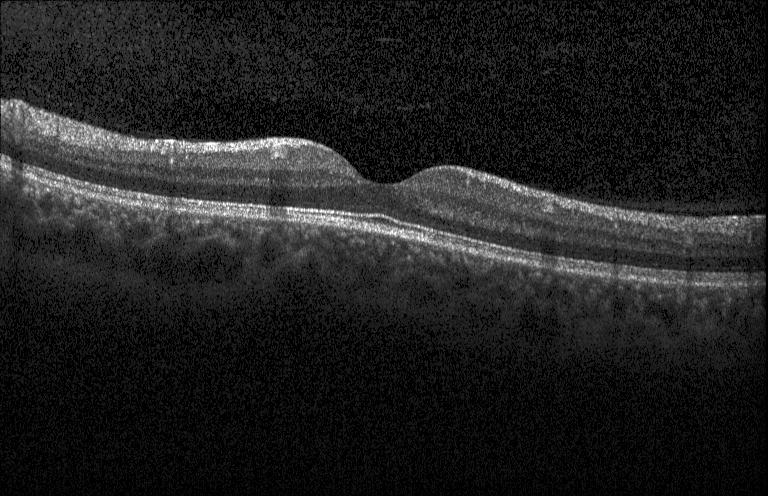 Spectral-domain optical coherence tomography, through the macula, retinal OCT B-scan
Finding: neither choroidal neovascularization, diabetic macular edema, nor drusen.